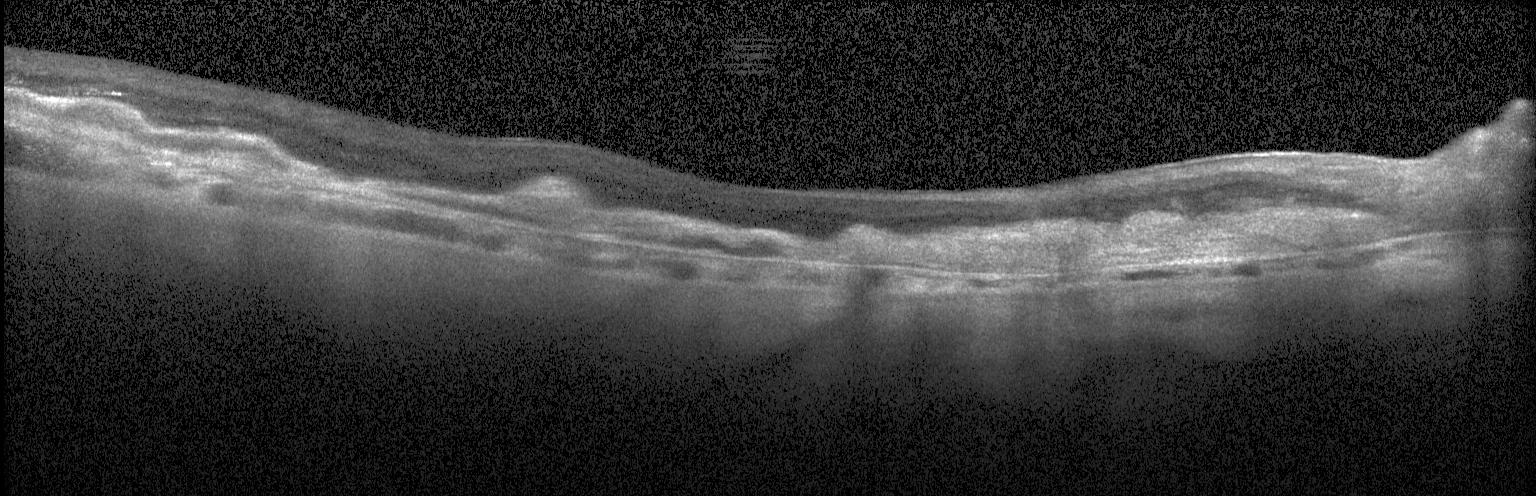
Finding: a choroidal neovascular membrane.